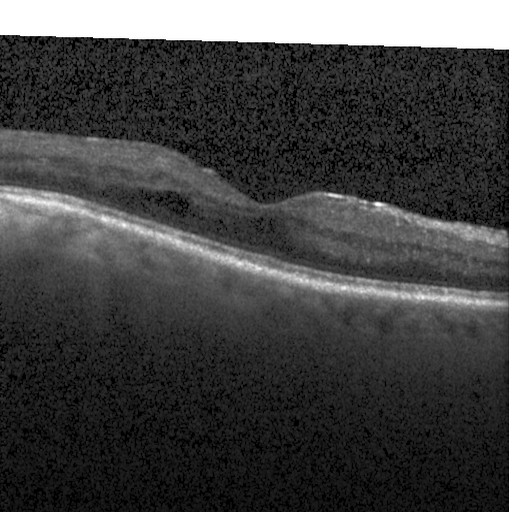

Finding: DME.